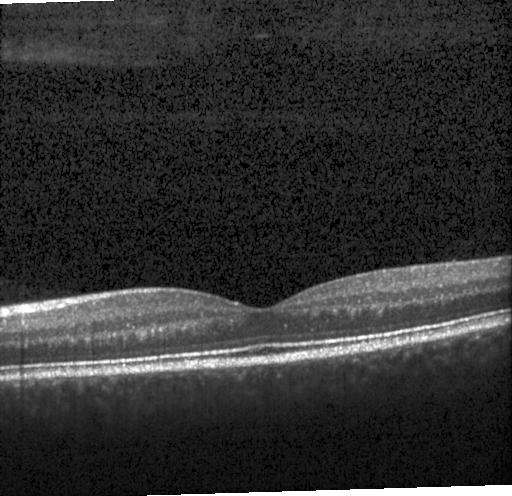
Optical coherence tomography scan — This B-scan demonstrates no choroidal neovascularization, no diabetic macular edema, and no drusen.